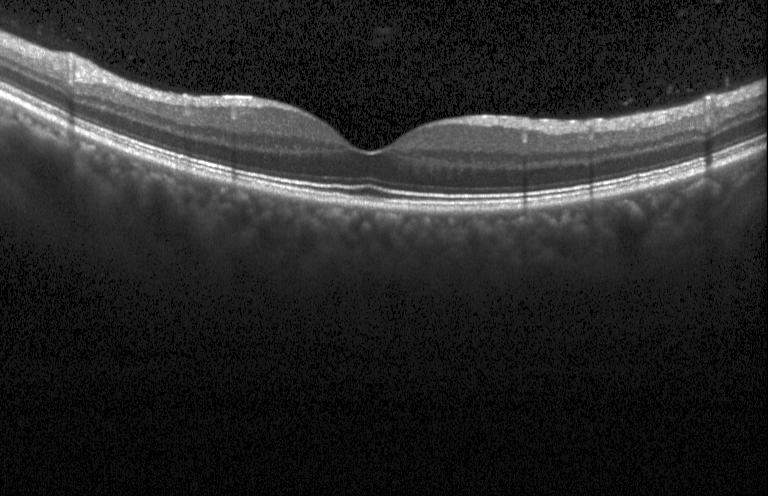
This B-scan demonstrates no evidence of CNV, DME, or drusen.